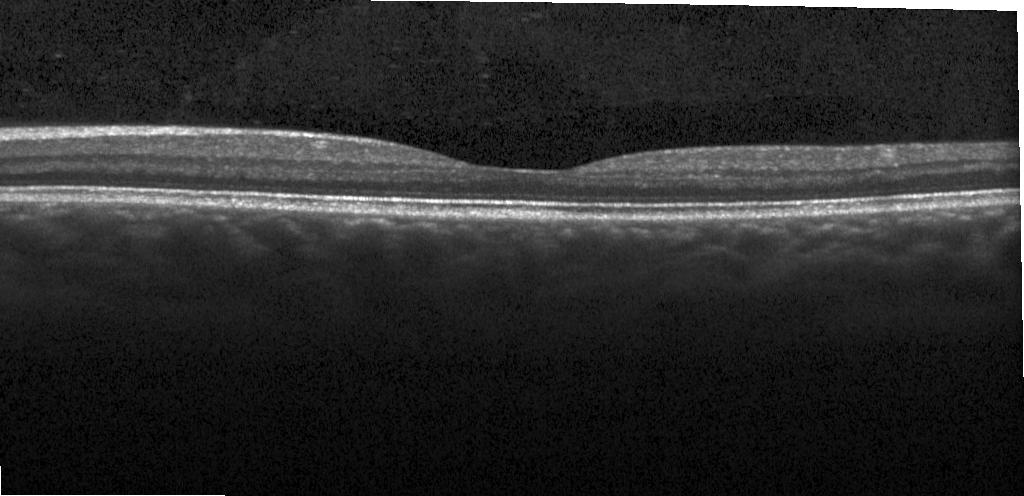 Optical coherence tomography scan · SD-OCT · horizontal scan through the fovea · Heidelberg Spectralis OCT system.
Dx: no evidence of choroidal neovascularization, diabetic macular edema, or drusen.